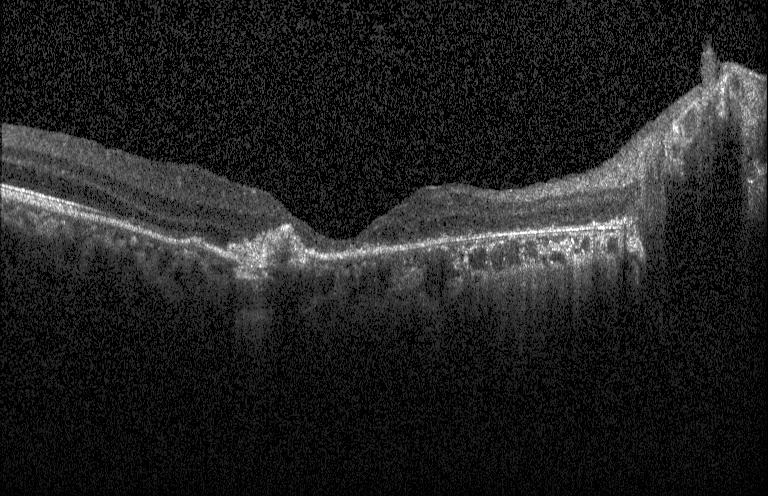
Impression: choroidal neovascularization.